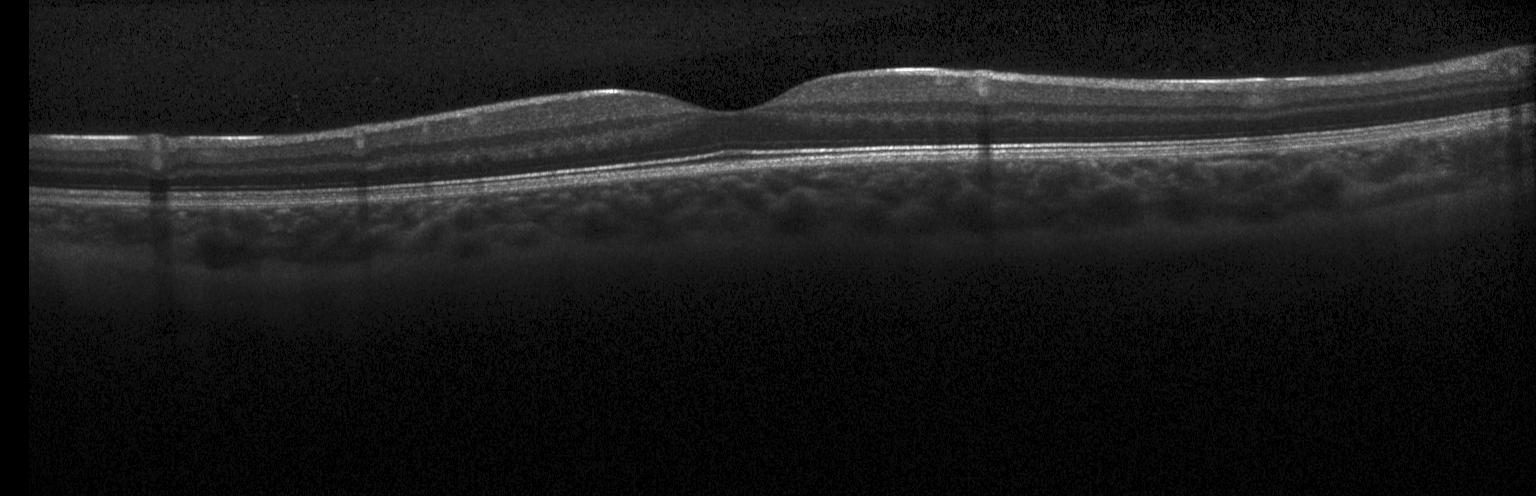 Acquired on a Heidelberg Spectralis · retinal OCT cross-section · SD-OCT — Impression: neither CNV, DME, nor drusen.